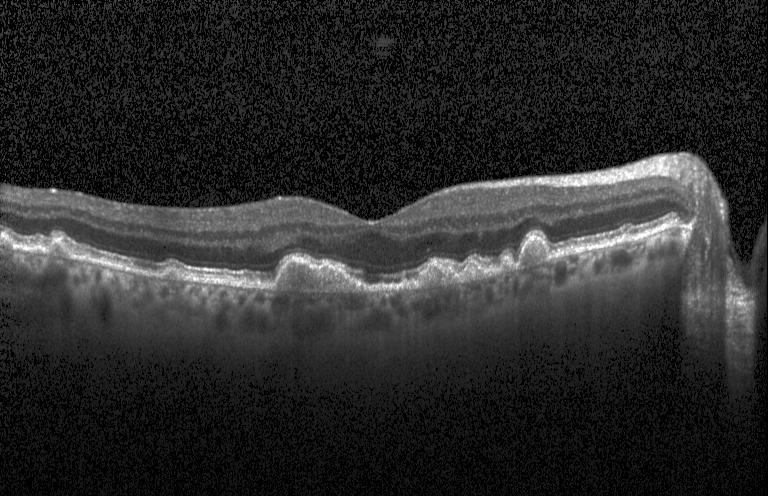
OCT scan showing sub-RPE drusenoid deposits.